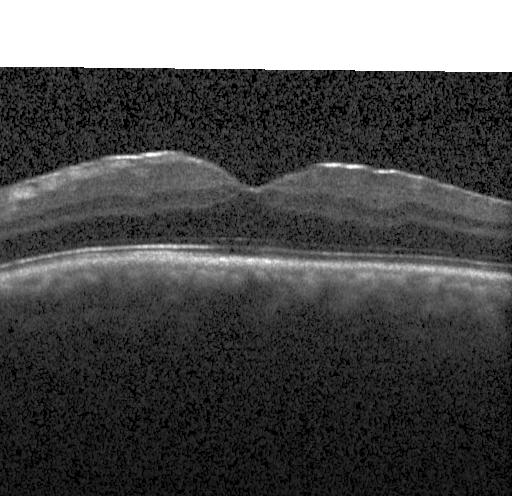
The scan shows no evidence of choroidal neovascularization, diabetic macular edema, or drusen.